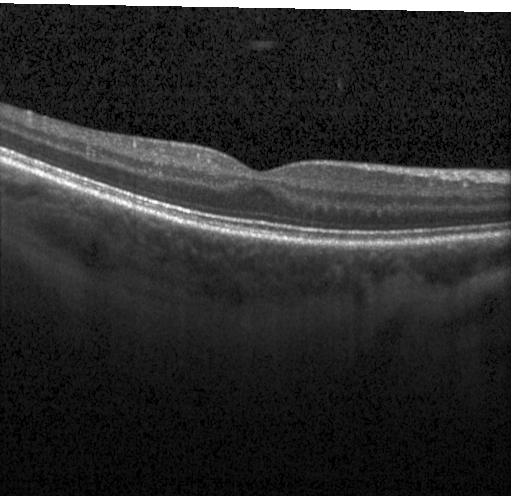

Spectral-domain optical coherence tomography. Horizontal scan through the fovea. Retinal OCT B-scan — Diagnosis: neither CNV, DME, nor drusen.